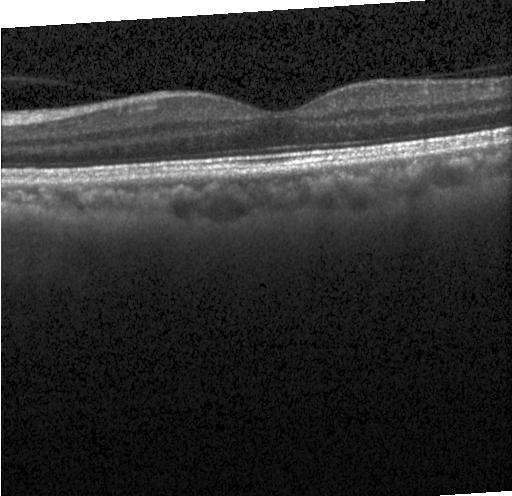 Optical coherence tomography scan. Centered on the fovea. Instrument: Heidelberg Spectralis — Diagnosis: neither CNV, DME, nor drusen.